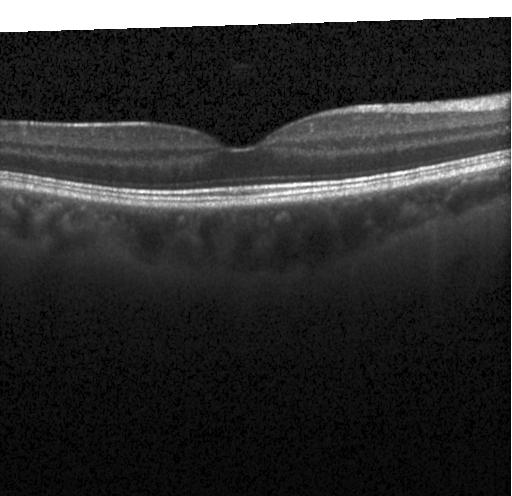 Spectral-domain optical coherence tomography, Heidelberg Spectralis, OCT B-scan. Diagnosis: no CNV, DME, or drusen.